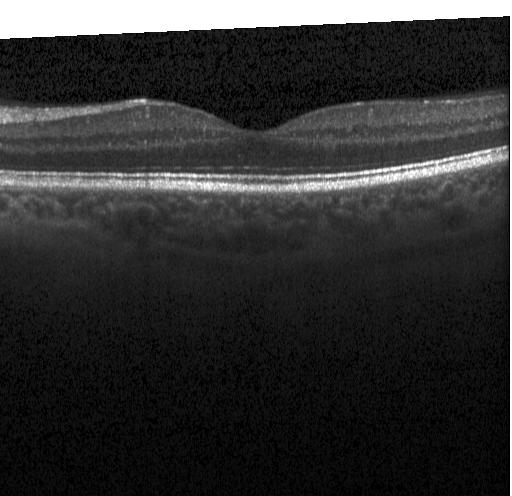 Assessment: no choroidal neovascularization, diabetic macular edema, or drusen.